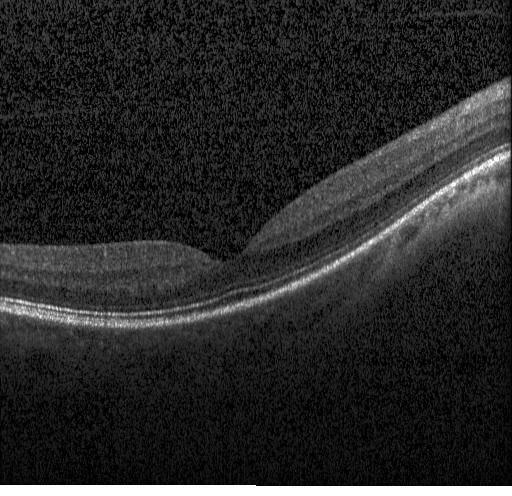
Retinal OCT cross-section
Impression: no CNV, no DME, and no drusen.